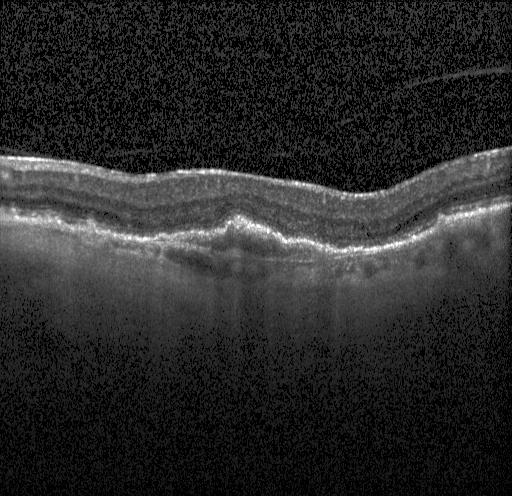 Macular scan · OCT line scan · spectral-domain optical coherence tomography — CNV.